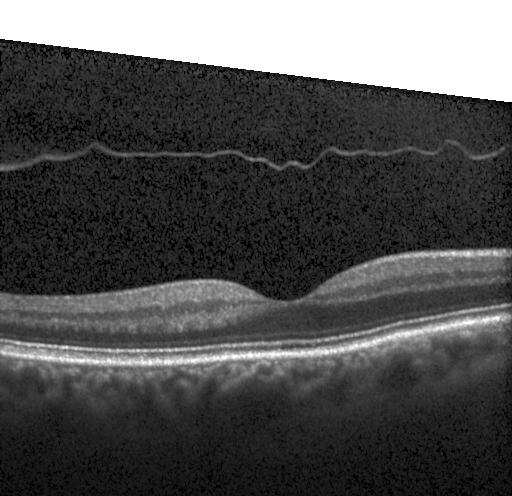

Dx: neither choroidal neovascularization, diabetic macular edema, nor drusen.